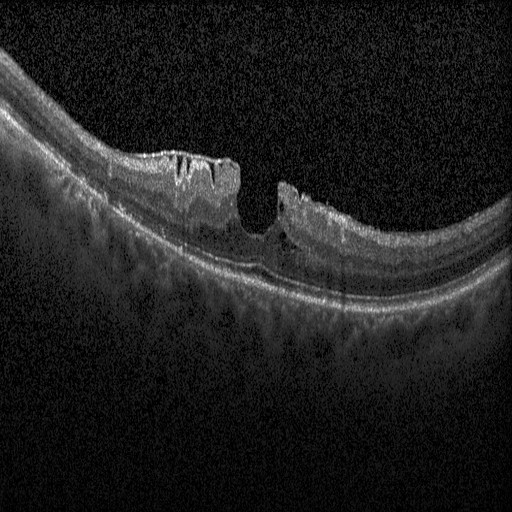

OCT scan showing DME.